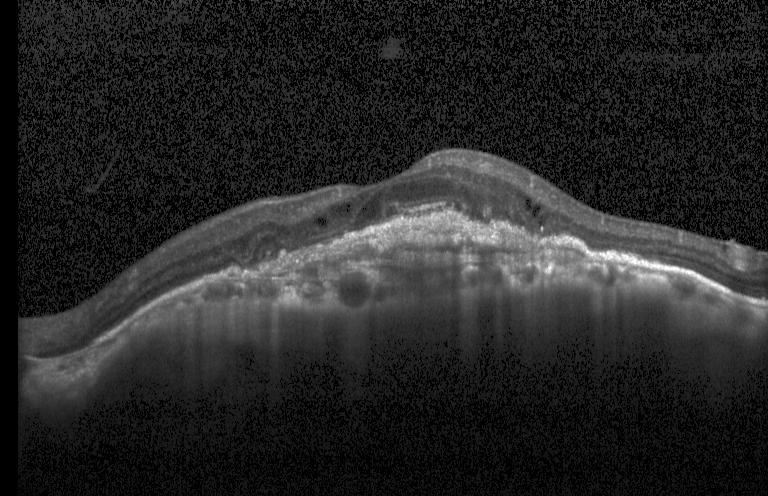
OCT B-scan. Impression: a choroidal neovascular membrane.